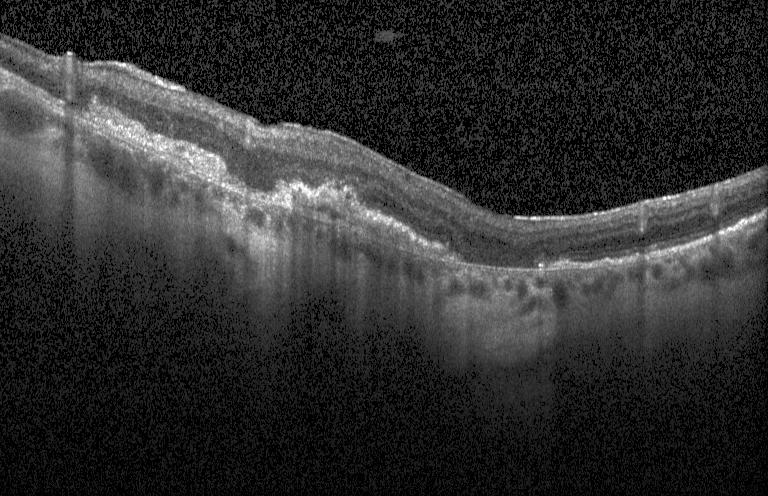
Optical coherence tomography B-scan — Impression: a choroidal neovascular membrane.